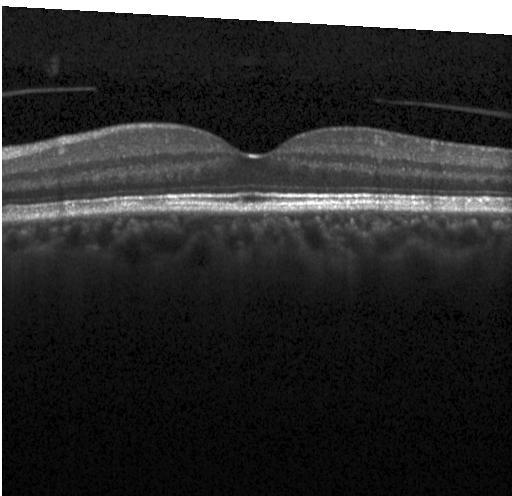 OCT scan showing no evidence of CNV, DME, or drusen.